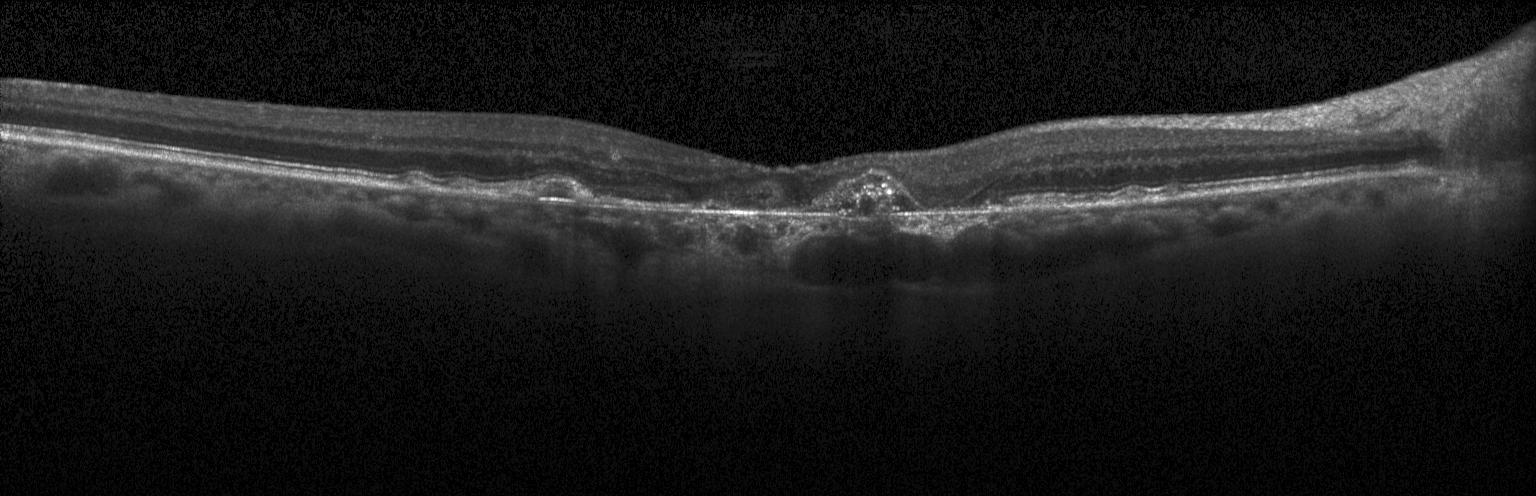

Heidelberg Spectralis; optical coherence tomography scan; SD-OCT; through the macula.
Diagnosis: CNV.